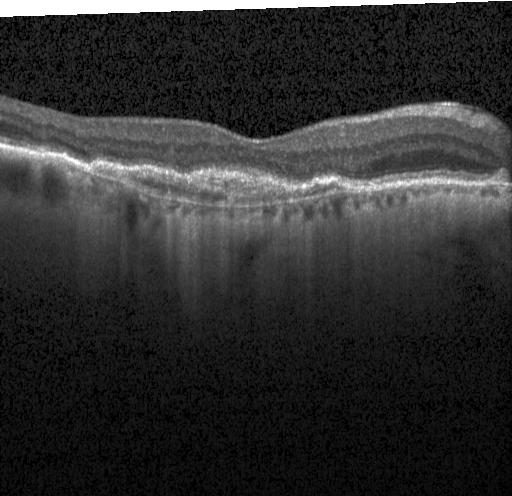 Optical coherence tomography scan. The scan shows a choroidal neovascular membrane.